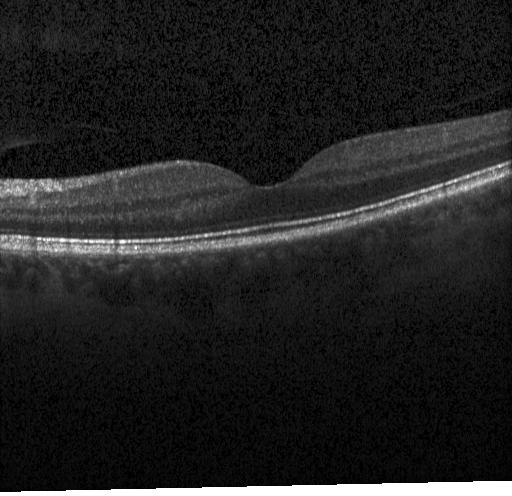

OCT scan showing no evidence of CNV, DME, or drusen.